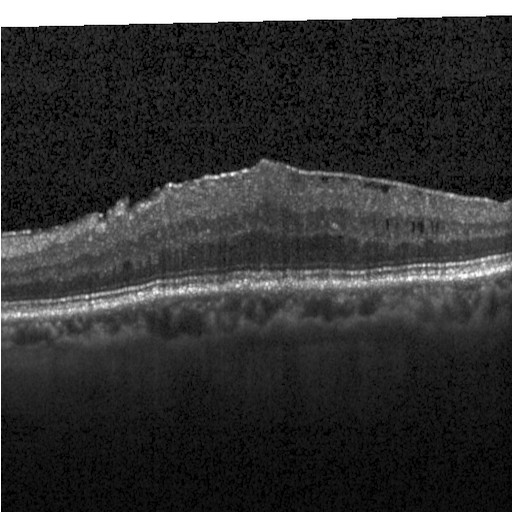

OCT scan showing diabetic macular edema.